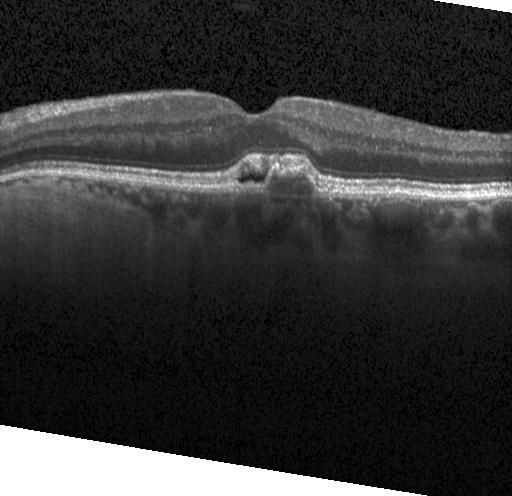

Spectral-domain OCT · OCT line scan · acquired on a Heidelberg Spectralis · horizontal scan through the fovea.
Assessment: a choroidal neovascular membrane.